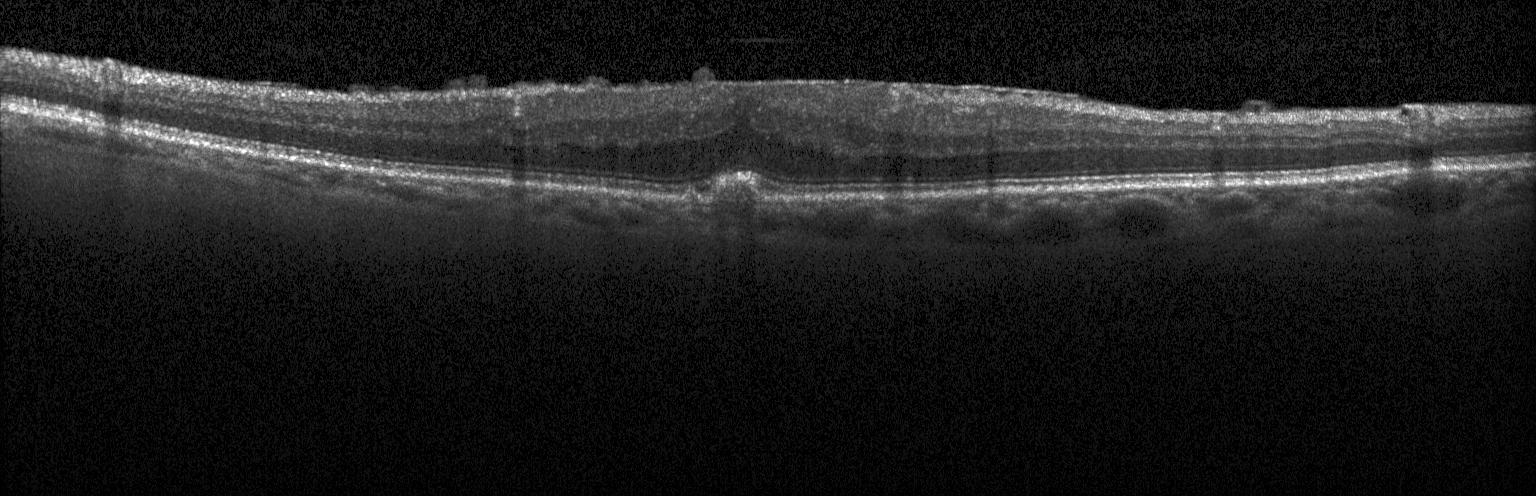
Centered on the fovea · OCT B-scan · Heidelberg Spectralis — Impression: drusen.